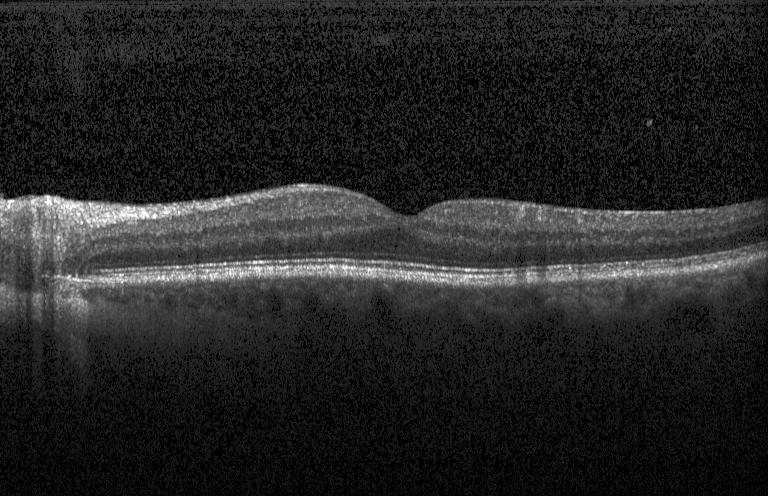

Spectral-domain optical coherence tomography, centered on the fovea, instrument: Heidelberg Spectralis, OCT line scan. No choroidal neovascularization, no diabetic macular edema, and no drusen.